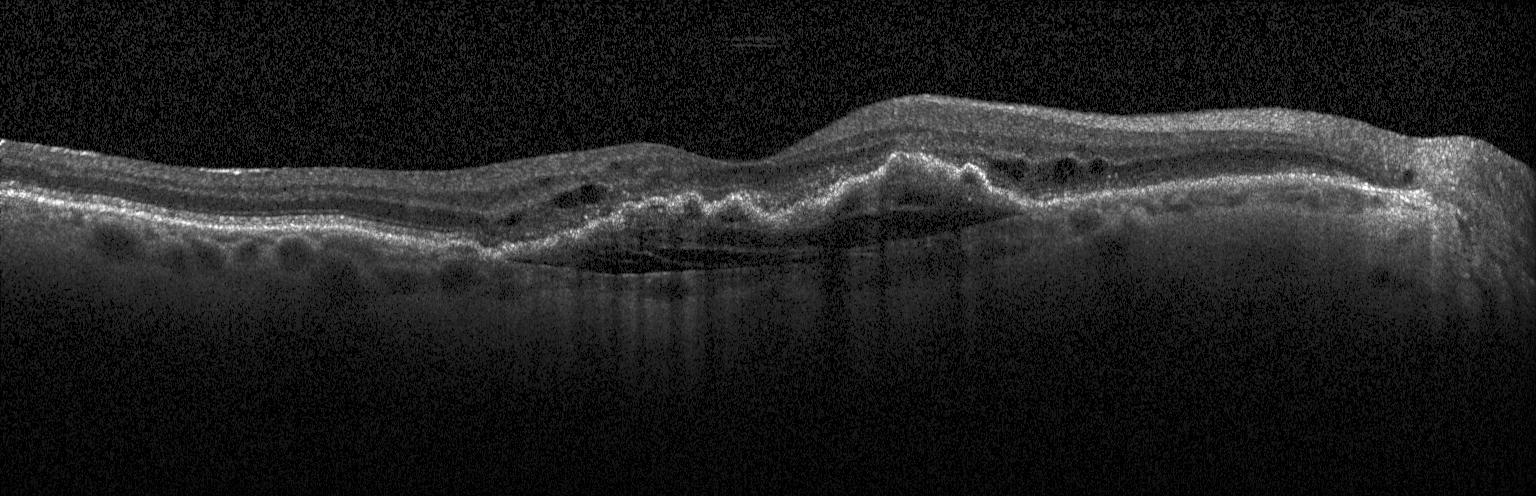
Spectral-domain optical coherence tomography; Heidelberg Spectralis OCT system; retinal OCT cross-section; through the macula.
The scan shows a choroidal neovascular membrane.